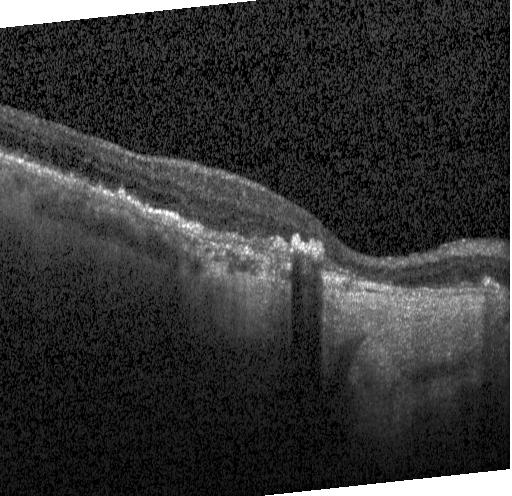

Finding: a choroidal neovascular membrane.